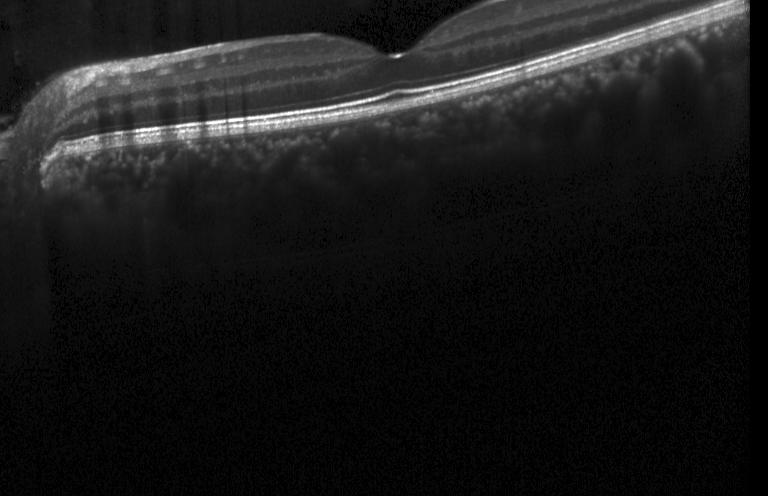
Heidelberg Spectralis. Centered on the fovea. SD-OCT. Optical coherence tomography B-scan.
This B-scan demonstrates neither choroidal neovascularization, diabetic macular edema, nor drusen.